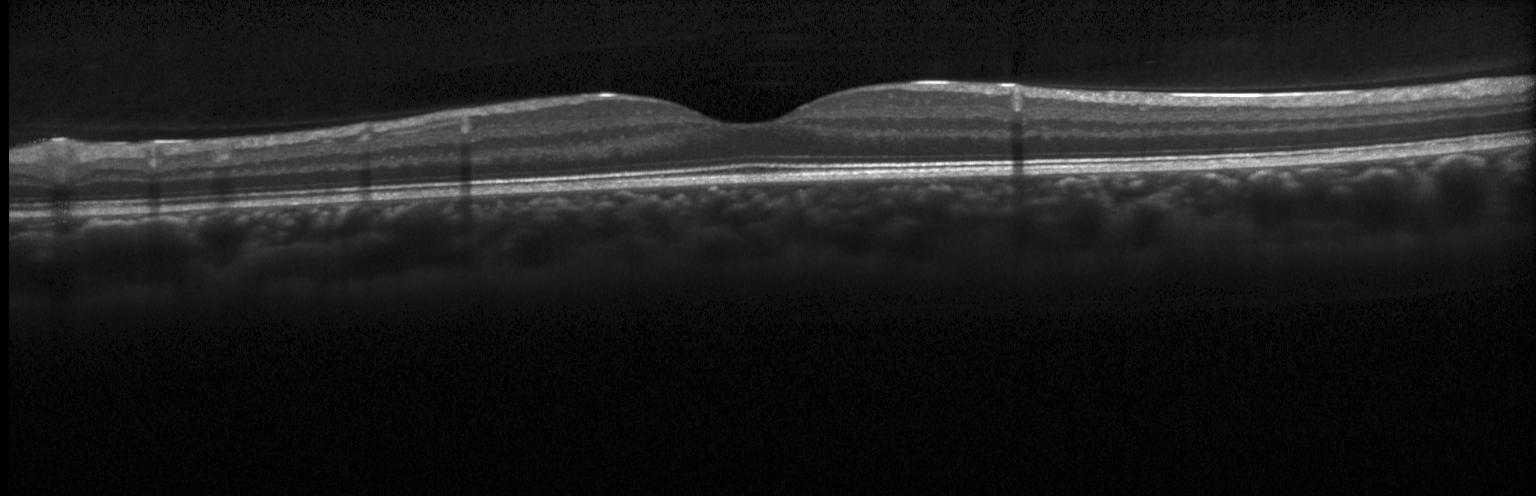

SD-OCT. Optical coherence tomography scan.
Diagnosis: no CNV, no DME, and no drusen.